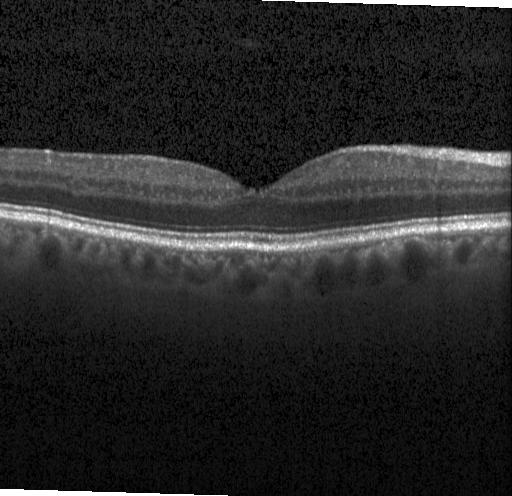 No evidence of choroidal neovascularization, diabetic macular edema, or drusen.